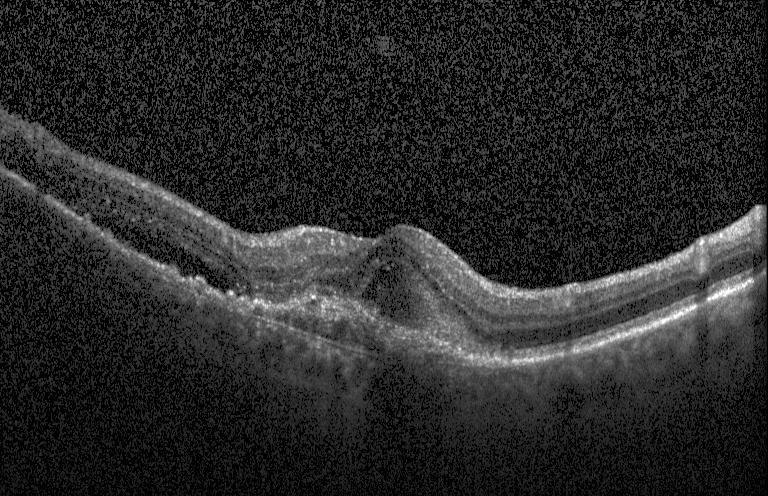
Assessment: a choroidal neovascular membrane.